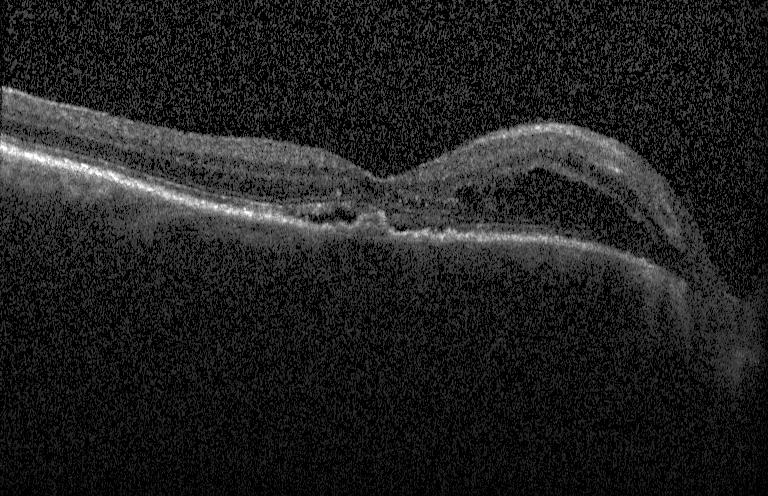

Retinal OCT B-scan. Impression: a choroidal neovascular membrane.